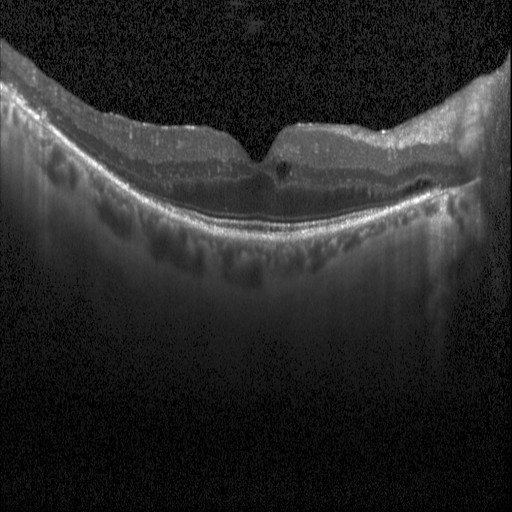 The scan shows DME.